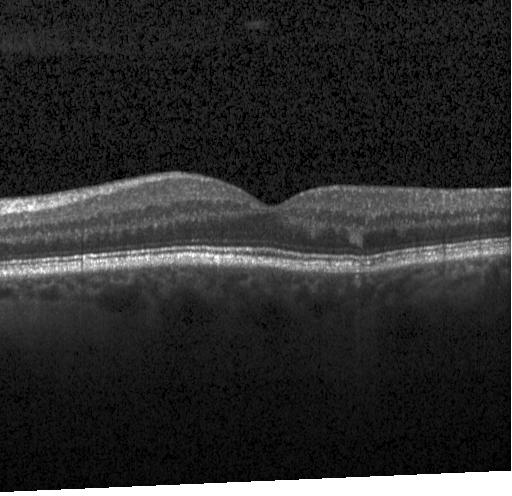

Assessment: no choroidal neovascularization, no diabetic macular edema, and no drusen.